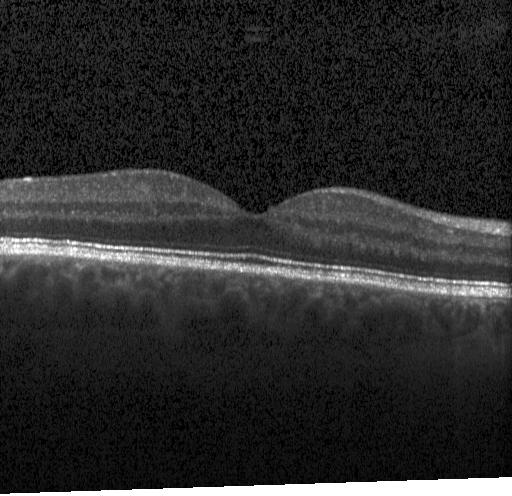 Diagnosis: no evidence of choroidal neovascularization, diabetic macular edema, or drusen.